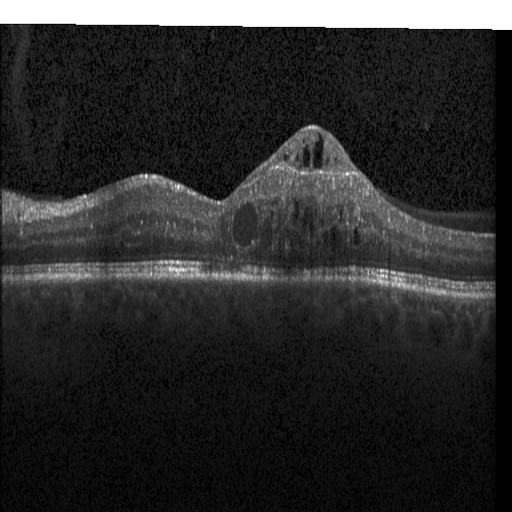
Spectral-domain optical coherence tomography · macular scan · acquired on a Heidelberg Spectralis · OCT line scan.
The scan shows DME.